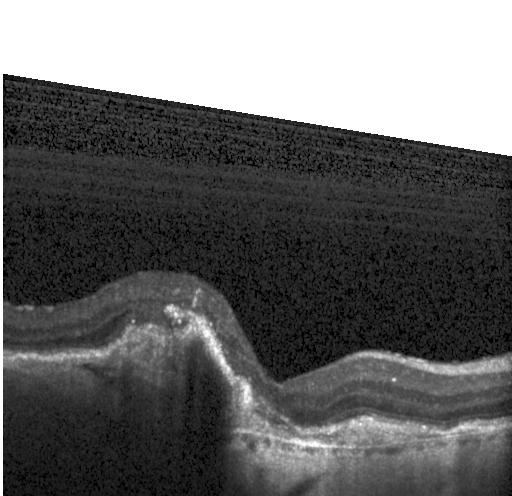

Assessment: a choroidal neovascular membrane.